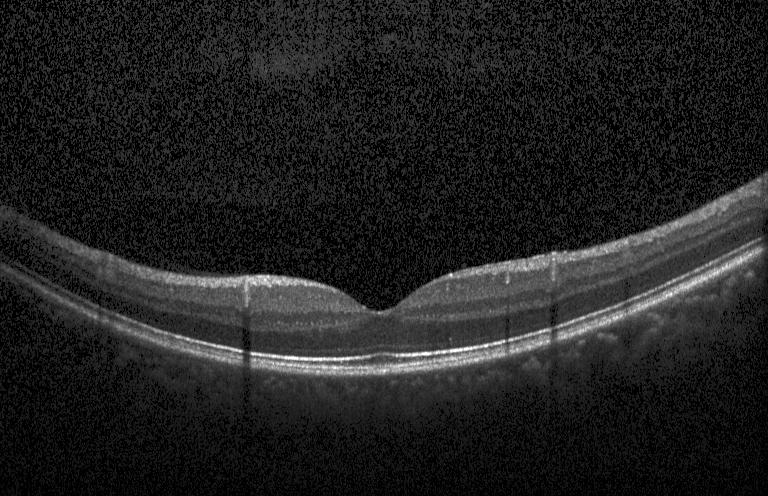
OCT B-scan
Impression: neither CNV, DME, nor drusen.